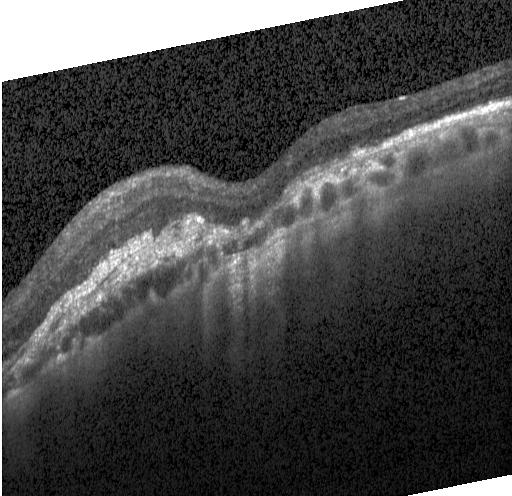
Retinal OCT cross-section, Heidelberg Spectralis, horizontal scan through the fovea
The scan shows a choroidal neovascular membrane.